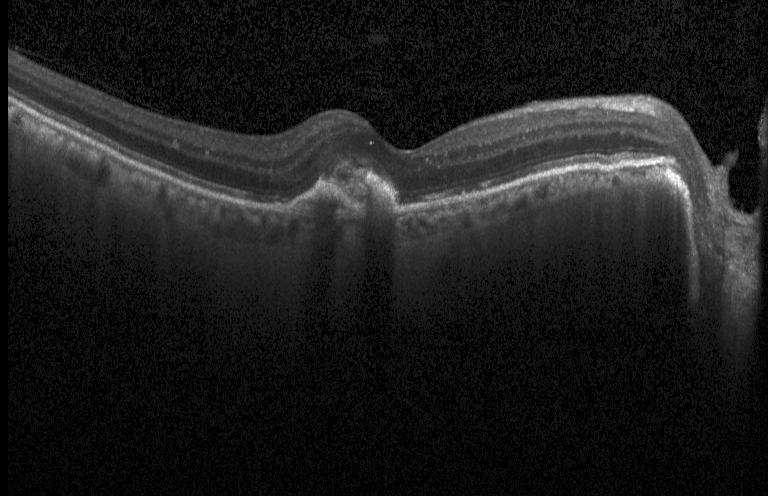 Fovea-centered. Retinal OCT B-scan. Heidelberg Spectralis OCT system. Impression: a choroidal neovascular membrane.